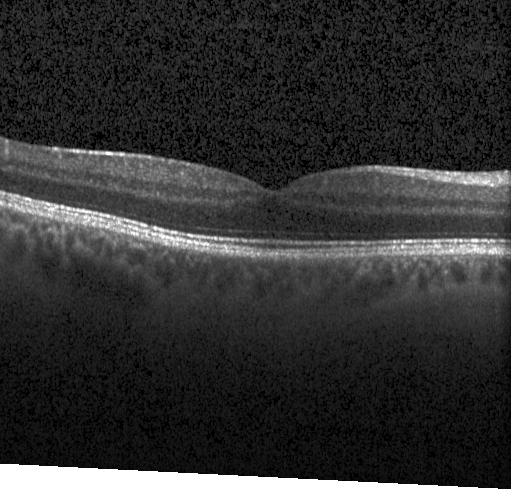

Optical coherence tomography scan. Macular scan. Spectral-domain OCT.
Finding: no CNV, DME, or drusen.